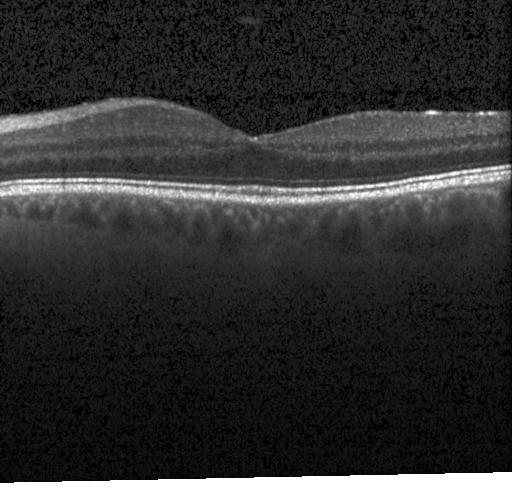 OCT B-scan. Instrument: Heidelberg Spectralis. SD-OCT
No choroidal neovascularization, diabetic macular edema, or drusen.